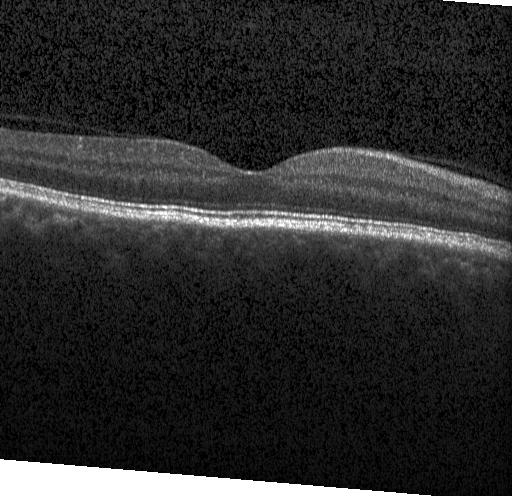 Optical coherence tomography scan
Diagnosis: no evidence of choroidal neovascularization, diabetic macular edema, or drusen.